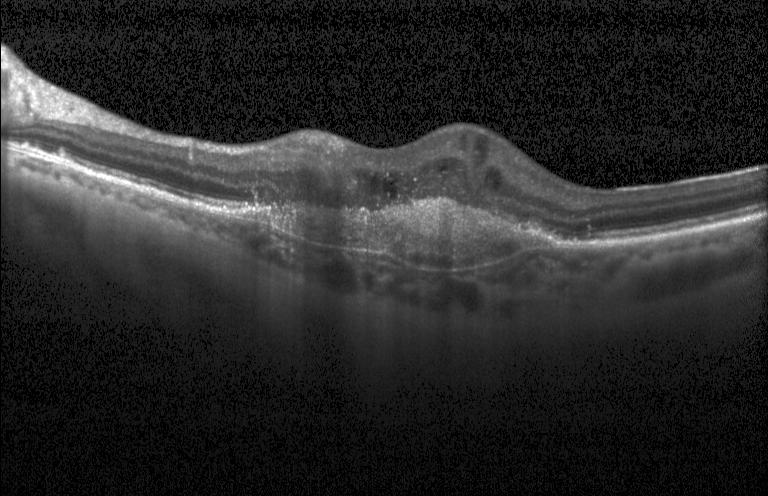

Horizontal scan through the fovea · optical coherence tomography B-scan · SD-OCT — Finding: choroidal neovascularization.